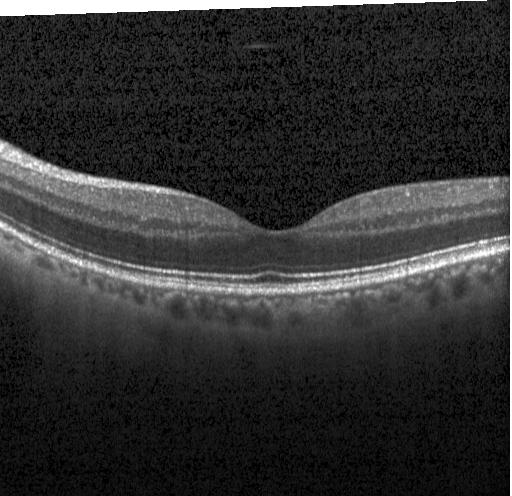

Retinal OCT B-scan · spectral-domain OCT · centered on the fovea — OCT finding: no evidence of CNV, DME, or drusen.